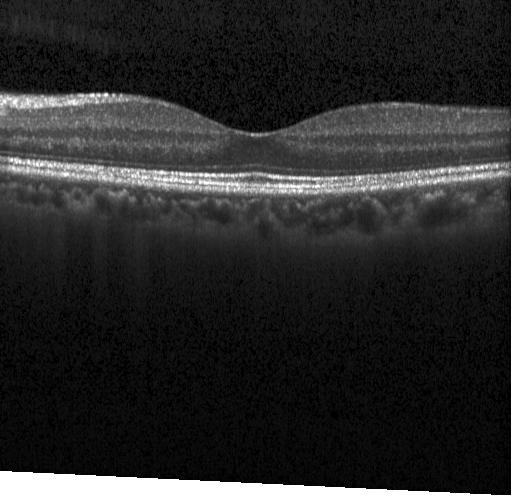

Retinal OCT cross-section showing no evidence of CNV, DME, or drusen.